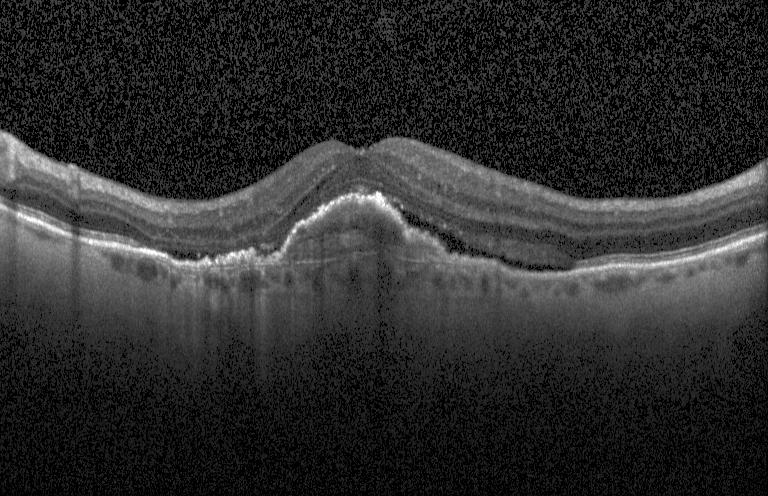 OCT B-scan showing a choroidal neovascular membrane.